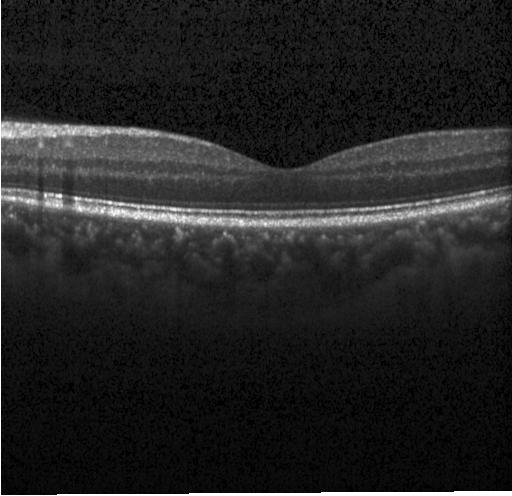
Fovea-centered. Retinal OCT cross-section. Impression: neither choroidal neovascularization, diabetic macular edema, nor drusen.